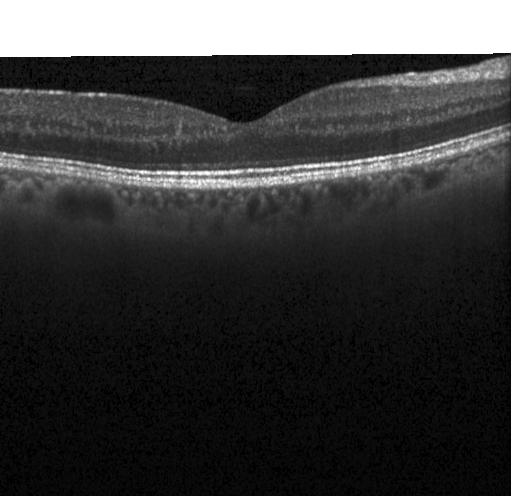 Optical coherence tomography B-scan
No CNV, DME, or drusen.